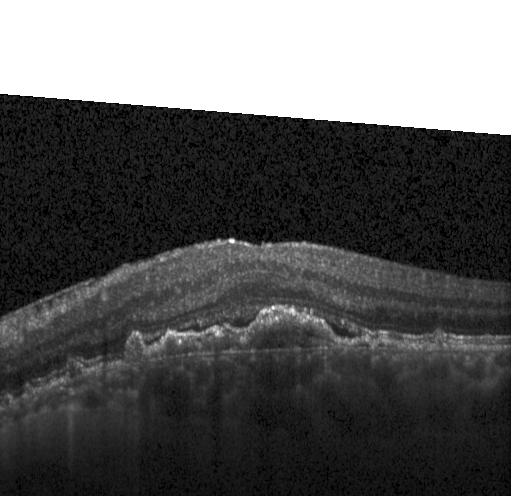
Macular OCT demonstrating CNV.